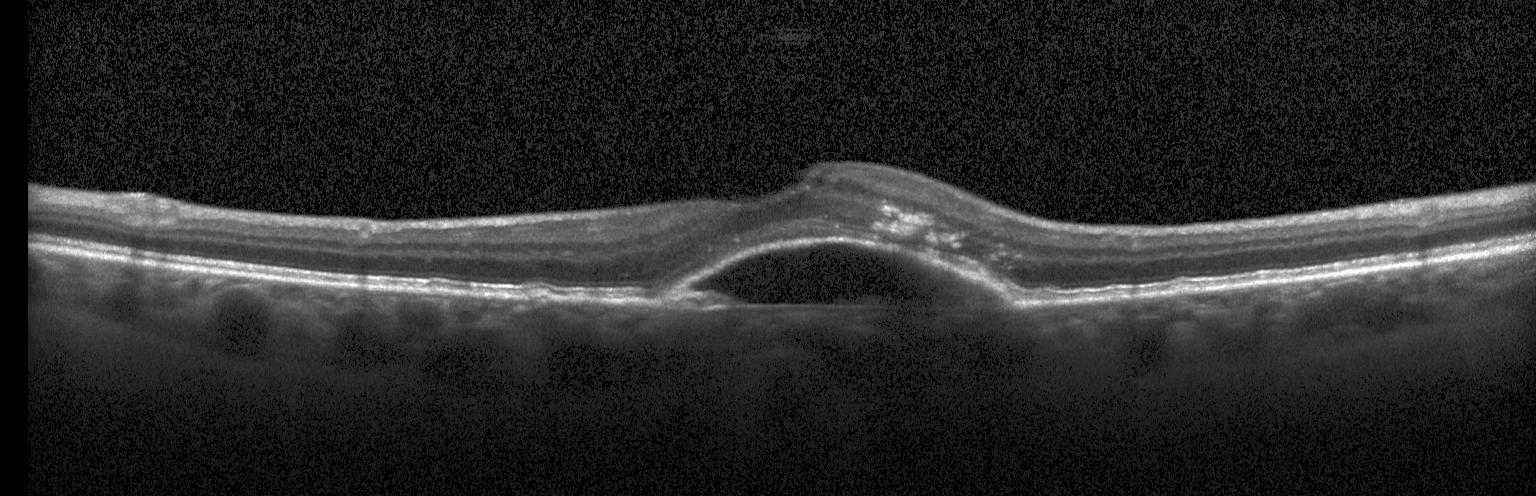 OCT B-scan · spectral-domain optical coherence tomography · macular scan
Macular OCT: a choroidal neovascular membrane.